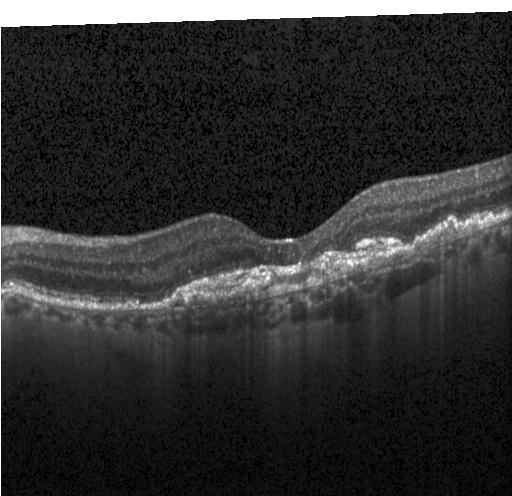
Spectral-domain OCT B-scan: a choroidal neovascular membrane.